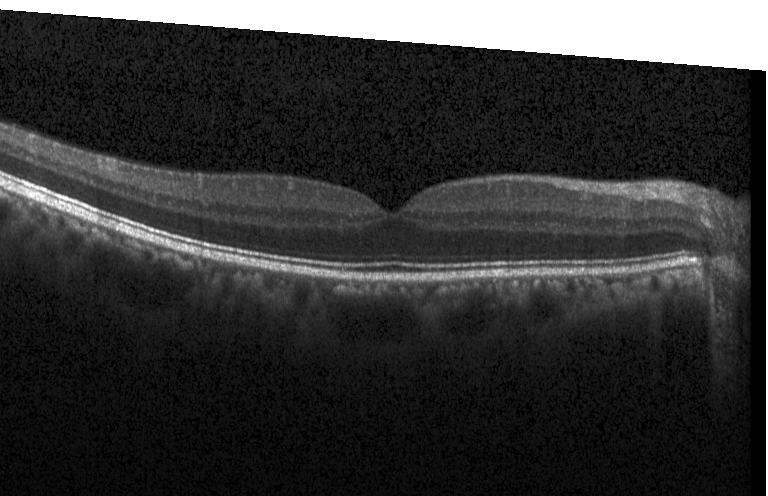

Macular scan; OCT B-scan.
Diagnosis: no choroidal neovascularization, no diabetic macular edema, and no drusen.